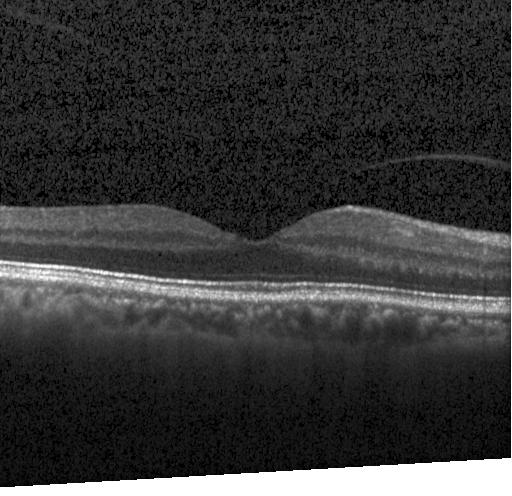

Centered on the fovea, Heidelberg Spectralis, spectral-domain OCT, optical coherence tomography scan
Finding: no CNV, DME, or drusen.